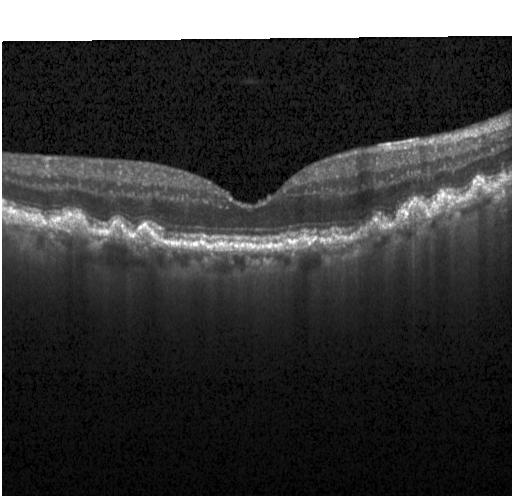

Instrument: Heidelberg Spectralis, retinal OCT B-scan, spectral-domain OCT, centered on the fovea.
Dx: sub-RPE drusenoid deposits.